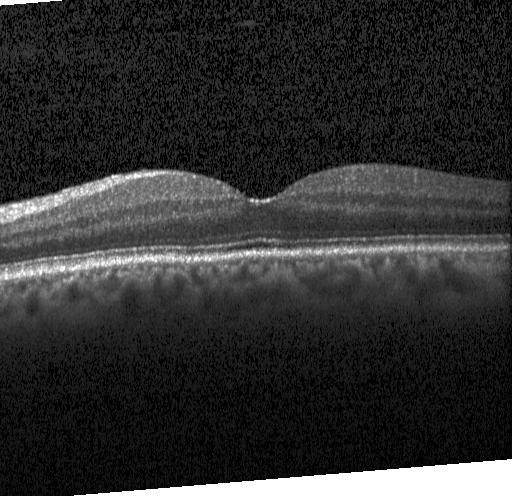

Assessment: no CNV, DME, or drusen.